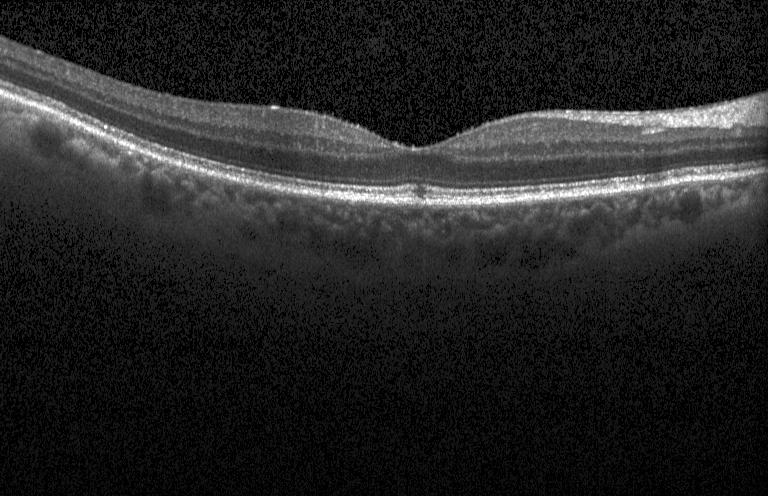

Impression: no CNV, no DME, and no drusen.